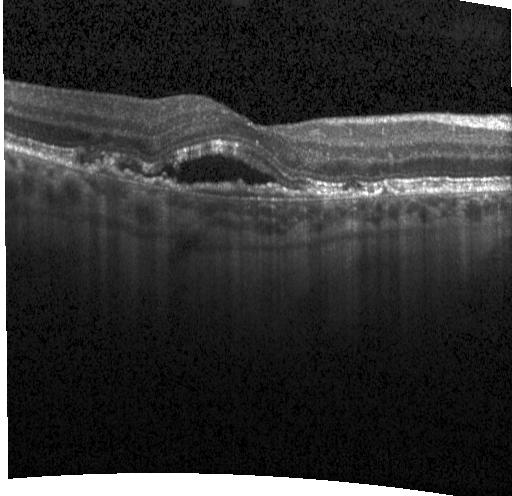

Assessment: CNV.